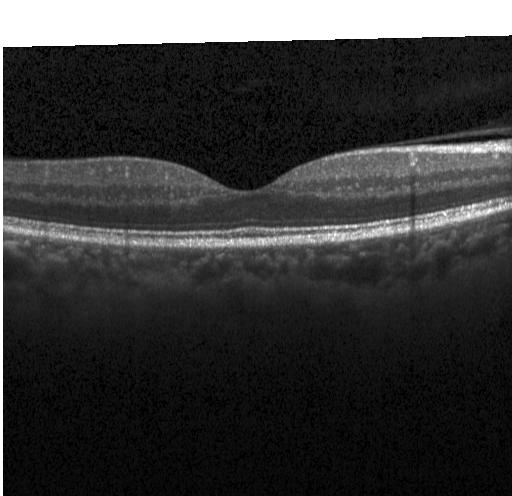
Spectral-domain OCT · optical coherence tomography scan · Heidelberg Spectralis OCT system. Assessment: neither choroidal neovascularization, diabetic macular edema, nor drusen.